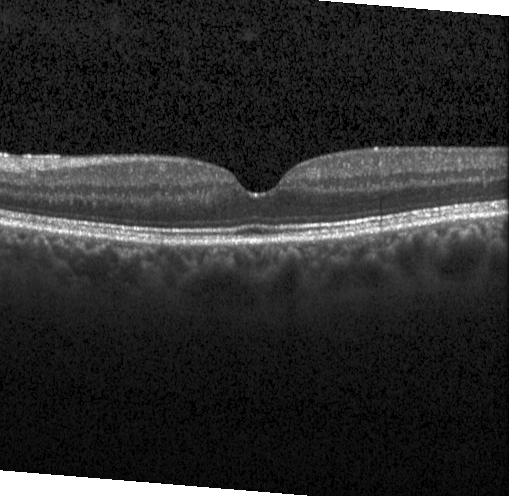
Heidelberg Spectralis, centered on the fovea, retinal OCT cross-section
The scan shows neither choroidal neovascularization, diabetic macular edema, nor drusen.